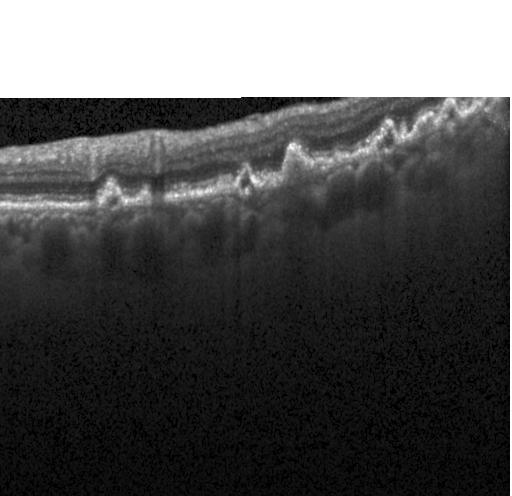

Heidelberg Spectralis, OCT line scan, spectral-domain OCT.
Finding: choroidal neovascularization (CNV).